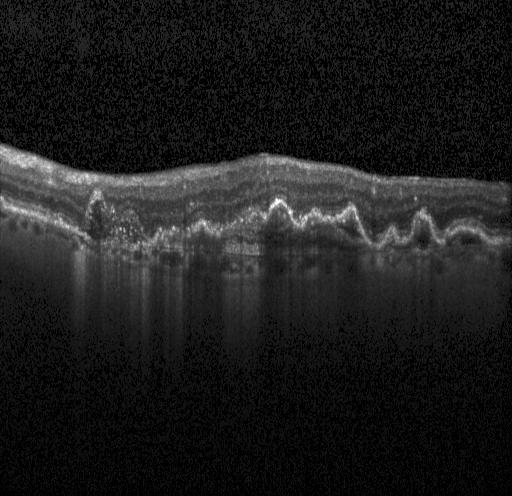

Retinal OCT B-scan — This B-scan demonstrates choroidal neovascularization.